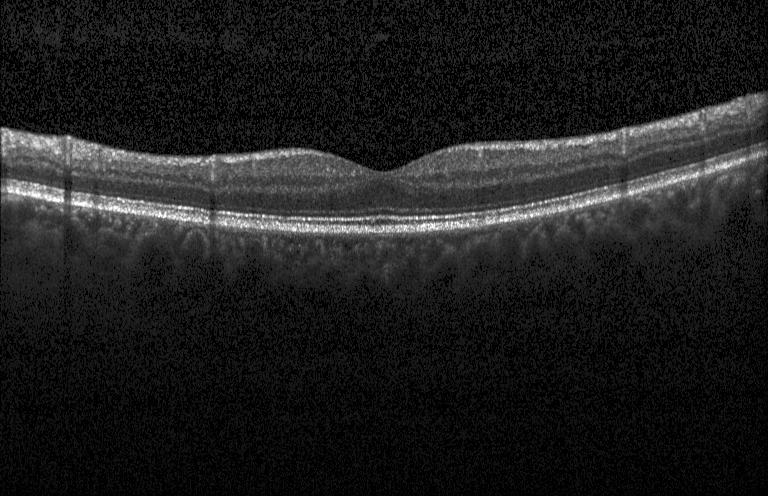

Optical coherence tomography B-scan, centered on the fovea.
Finding: no choroidal neovascularization, diabetic macular edema, or drusen.